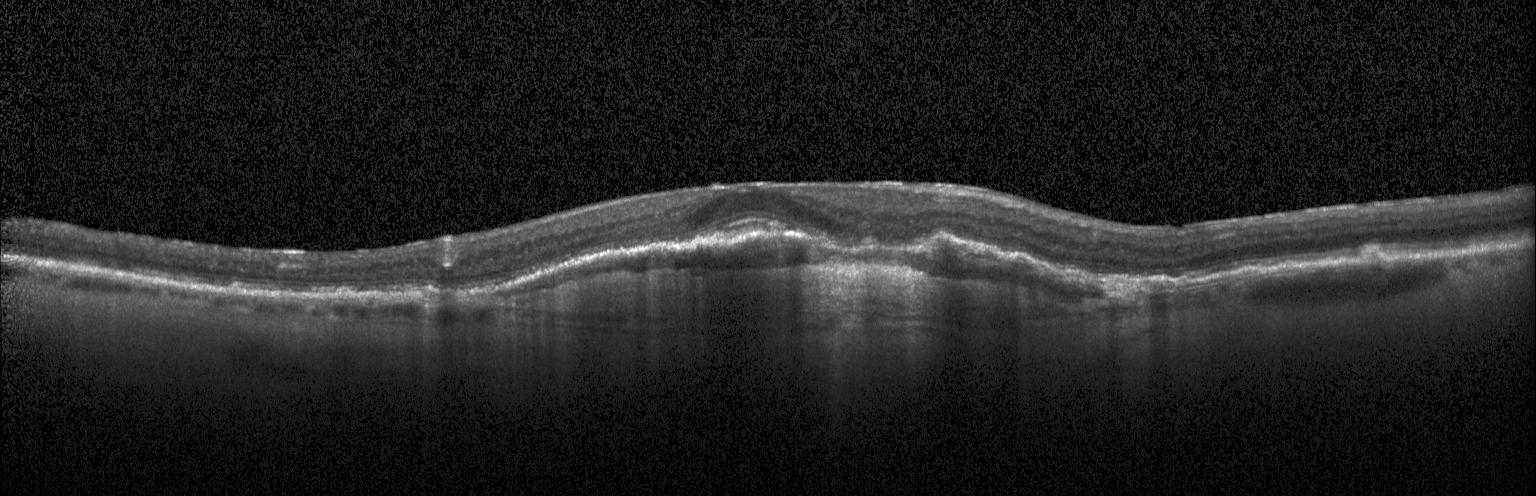

SD-OCT; optical coherence tomography B-scan; through the macula. Diagnosis: a choroidal neovascular membrane.